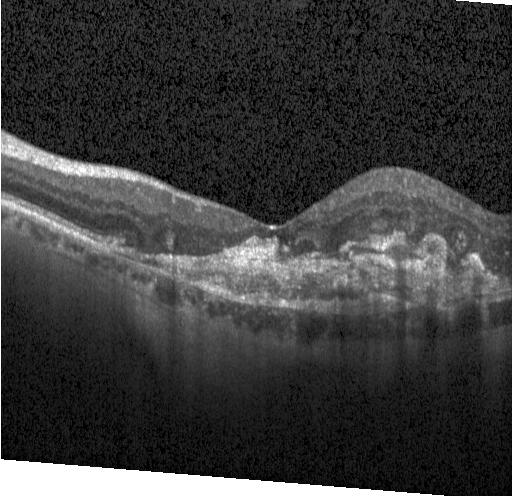
OCT line scan; through the macula; Heidelberg Spectralis OCT system. CNV.